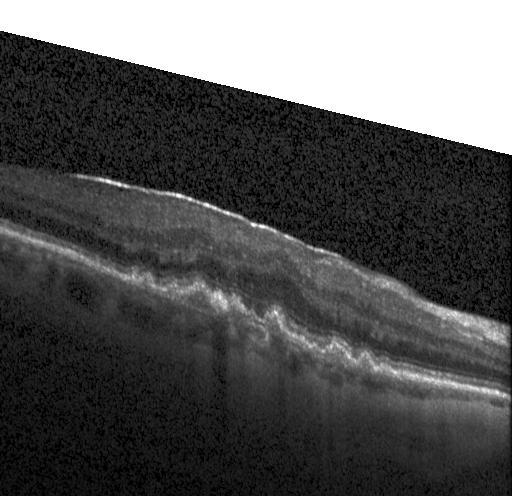 Impression: multiple drusen.